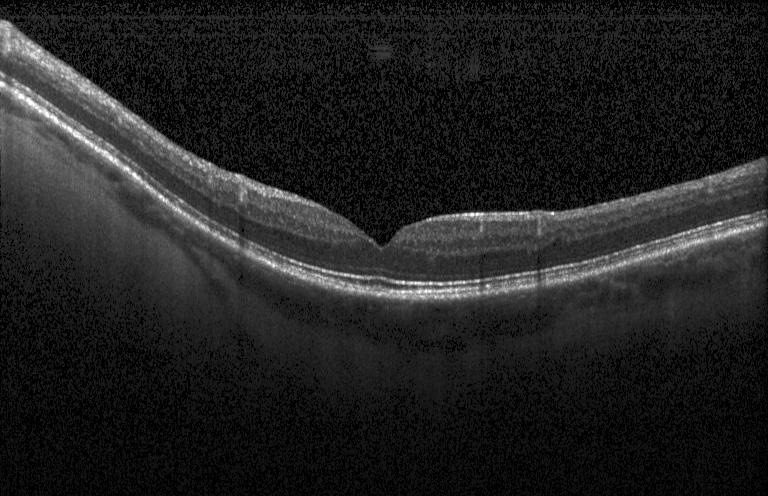
OCT B-scan; spectral-domain optical coherence tomography. Impression: no CNV, no DME, and no drusen.